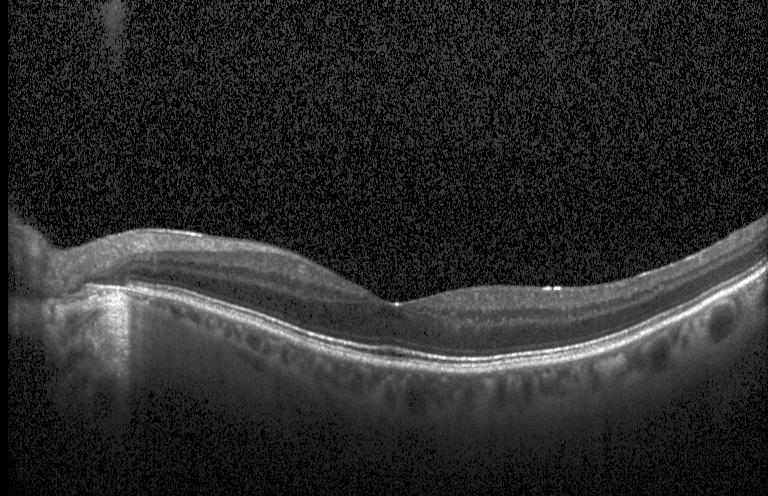

Instrument: Heidelberg Spectralis. Through the macula. SD-OCT. Optical coherence tomography scan — Diagnosis: no choroidal neovascularization, no diabetic macular edema, and no drusen.